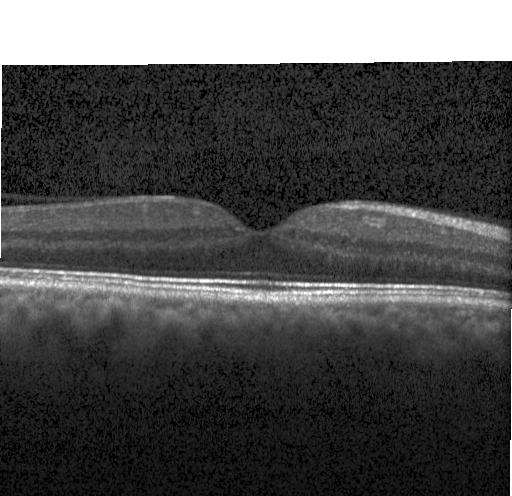 Retinal OCT cross-section, instrument: Heidelberg Spectralis, spectral-domain OCT, fovea-centered — Impression: no CNV, DME, or drusen.